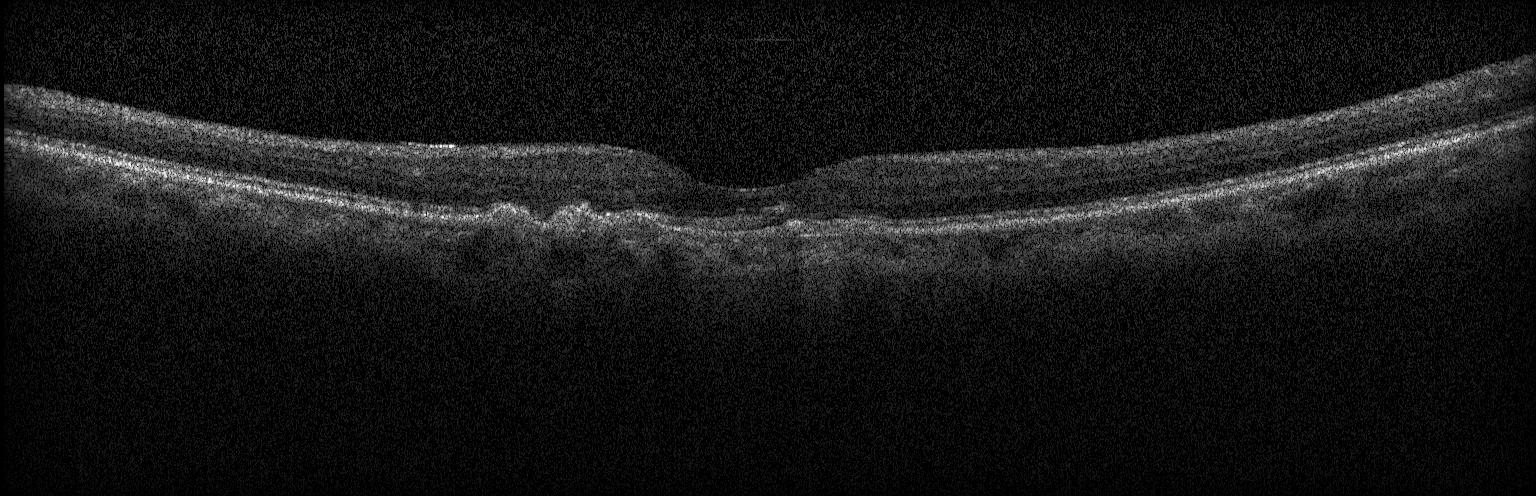 Dx: choroidal neovascularization.